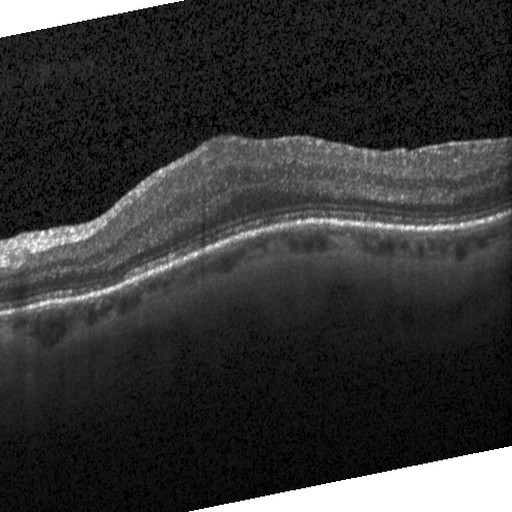
Retinal OCT B-scan
Diabetic macular edema (DME).